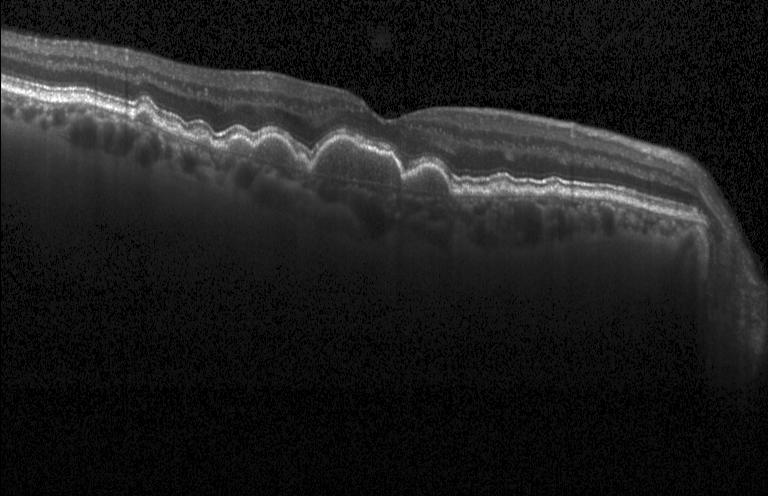 Finding: sub-RPE drusenoid deposits.